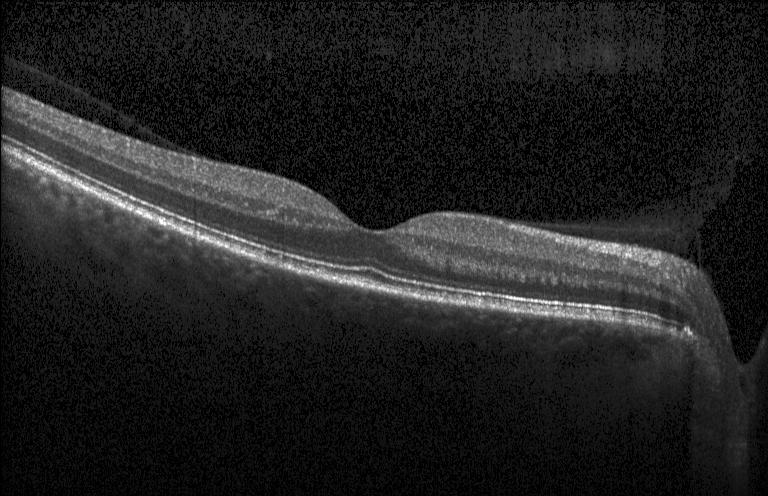 Optical coherence tomography scan. Through the macula. Heidelberg Spectralis. Spectral-domain optical coherence tomography.
Finding: neither CNV, DME, nor drusen.